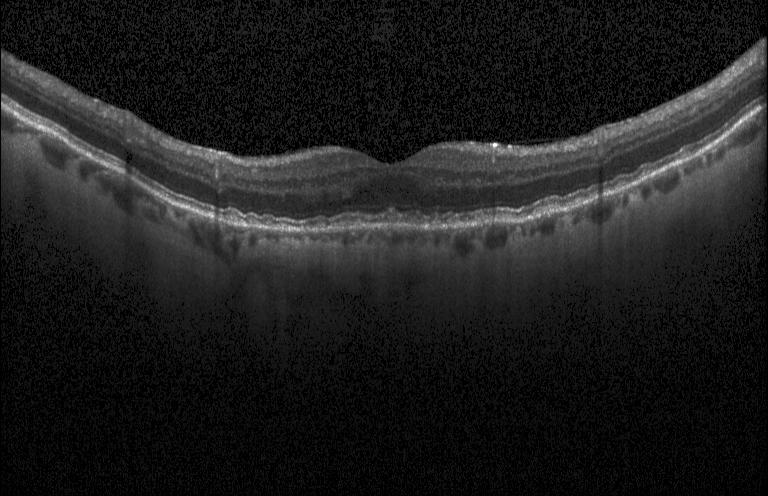 Optical coherence tomography scan; acquired on a Heidelberg Spectralis; fovea-centered. Macular OCT: multiple drusen.